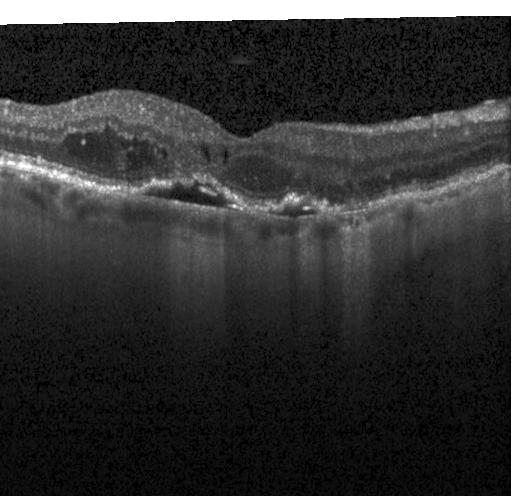
Retinal OCT B-scan.
This B-scan demonstrates CNV.